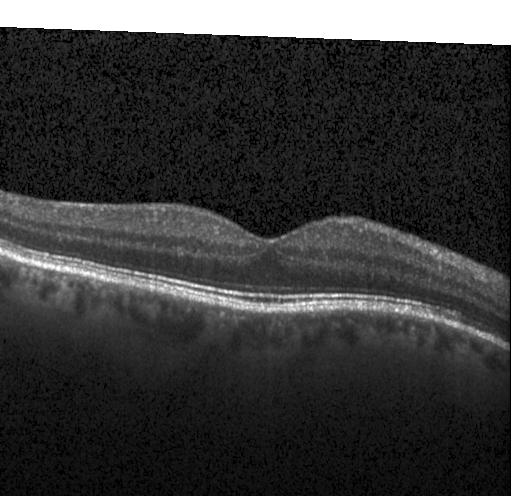
Retinal OCT cross-section showing no evidence of choroidal neovascularization, diabetic macular edema, or drusen.